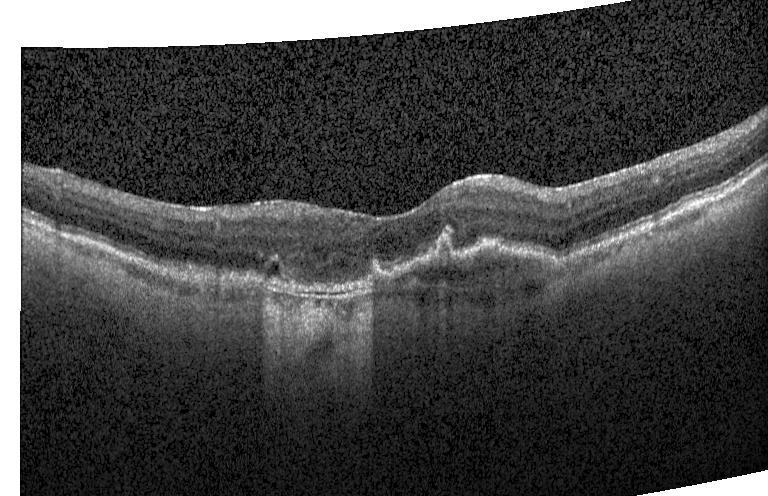 Macular scan · OCT B-scan · spectral-domain OCT.
OCT finding: choroidal neovascularization (CNV).